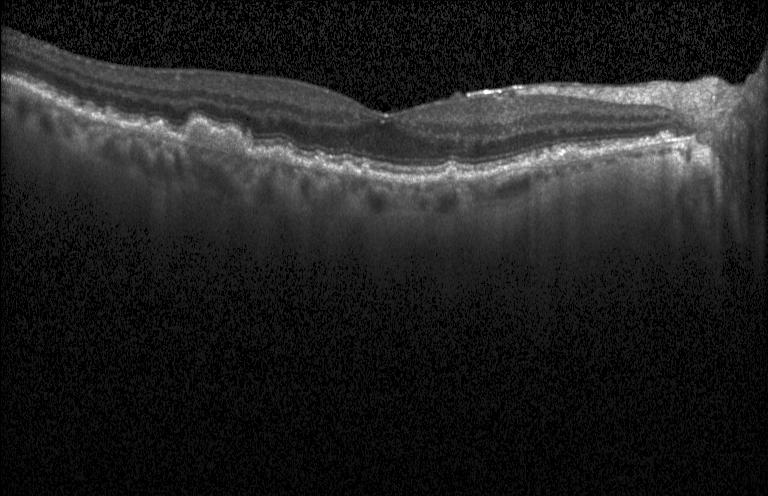

Optical coherence tomography scan.
Finding: sub-RPE drusenoid deposits.